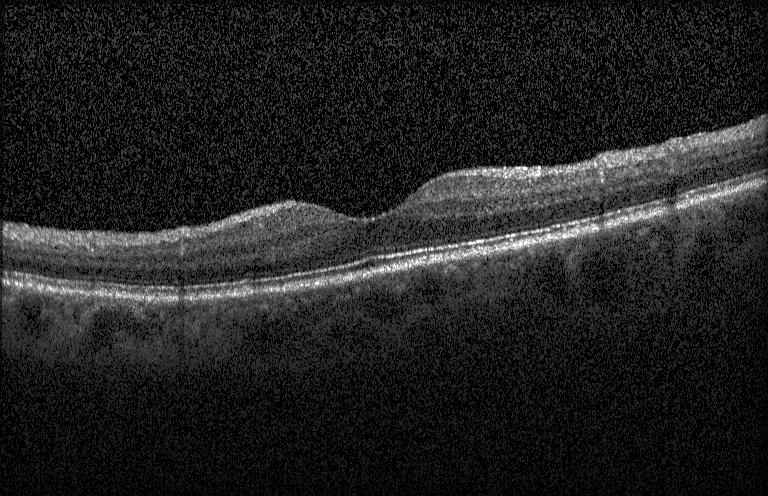 Spectral-domain optical coherence tomography, optical coherence tomography B-scan.
Finding: no choroidal neovascularization, no diabetic macular edema, and no drusen.